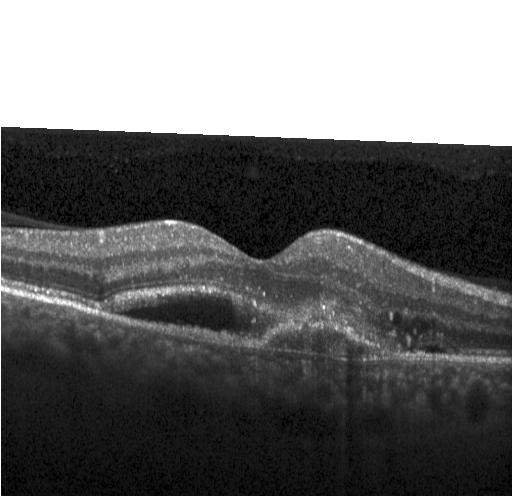

OCT finding: a choroidal neovascular membrane.